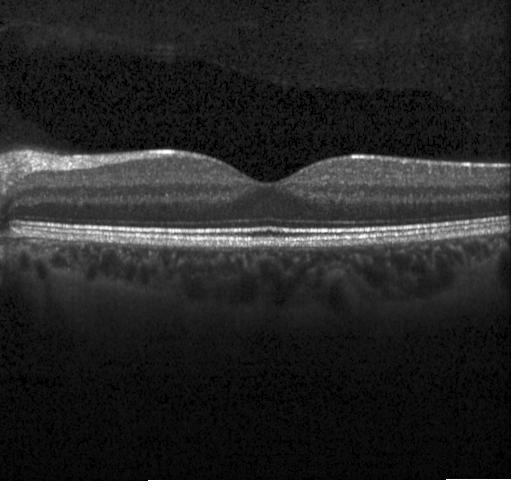

Spectral-domain OCT. Retinal OCT B-scan. Acquired on a Heidelberg Spectralis
Neither CNV, DME, nor drusen.